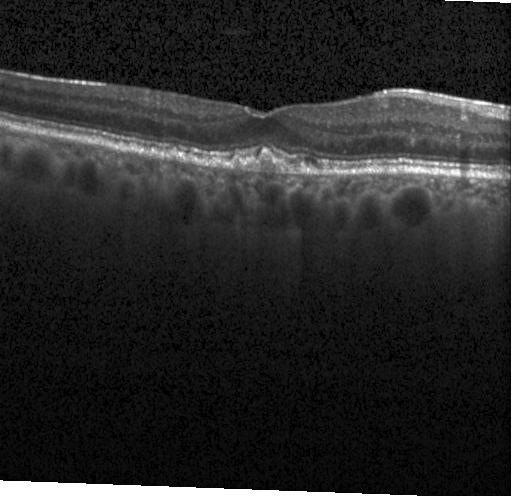 SD-OCT, optical coherence tomography B-scan, acquired on a Heidelberg Spectralis. Multiple drusen.